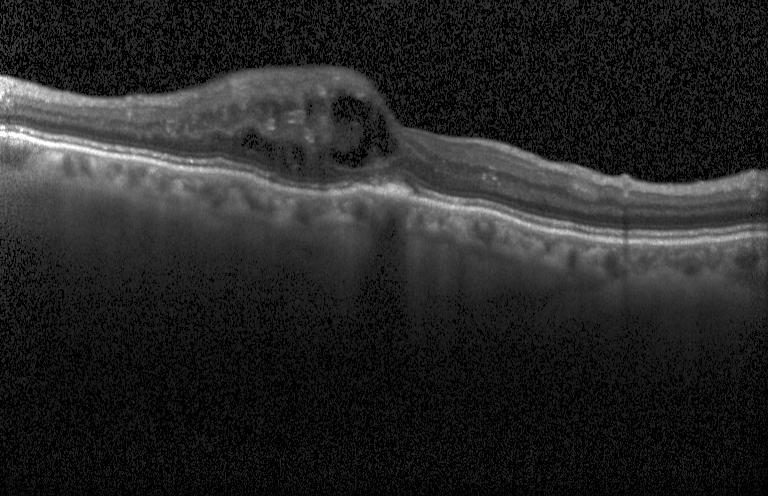
SD-OCT. Optical coherence tomography B-scan. Instrument: Heidelberg Spectralis
Impression: DME.